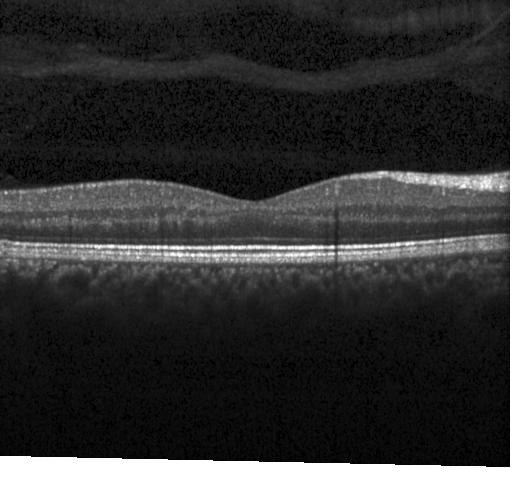 Spectral-domain OCT B-scan: no evidence of choroidal neovascularization, diabetic macular edema, or drusen.